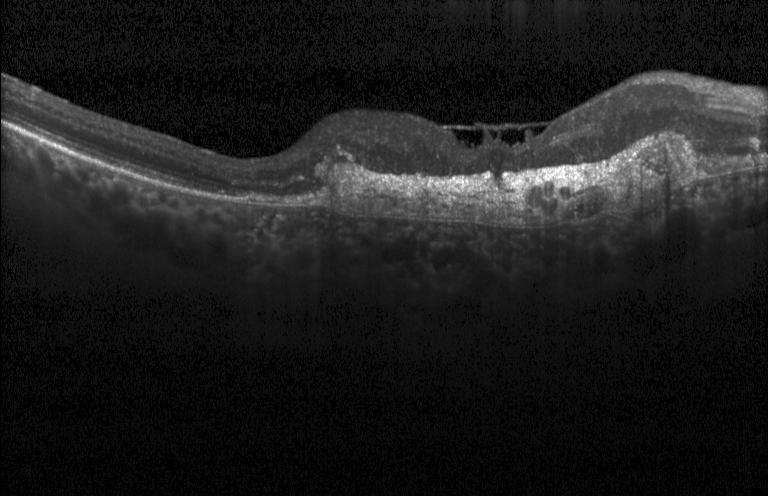
Acquired on a Heidelberg Spectralis, retinal OCT cross-section. Assessment: a choroidal neovascular membrane.